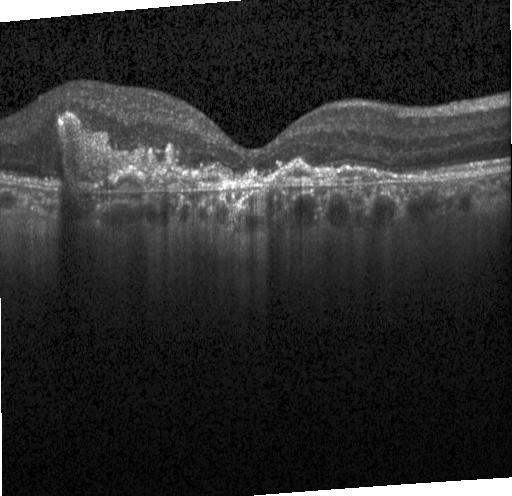 Retinal OCT cross-section, Heidelberg Spectralis — Assessment: a choroidal neovascular membrane.